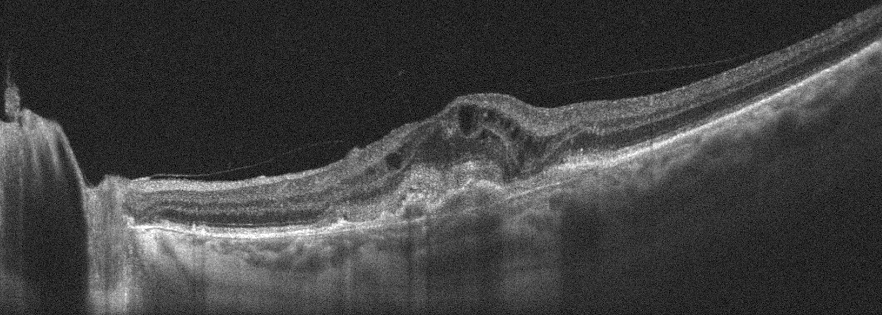 OCT B-scan; left eye. The scan shows AMD.